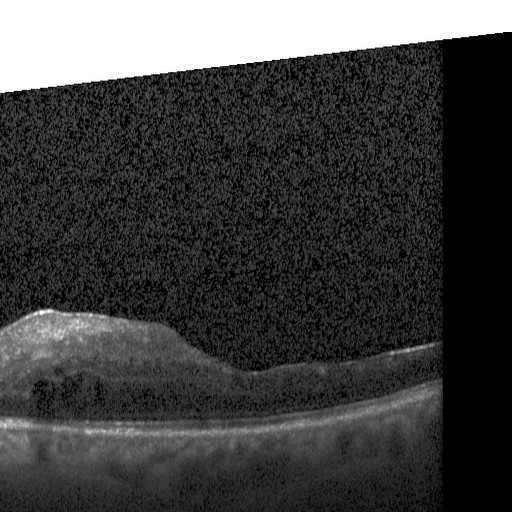

Instrument: Heidelberg Spectralis. Retinal OCT cross-section. Macular scan. Finding: diabetic macular edema.